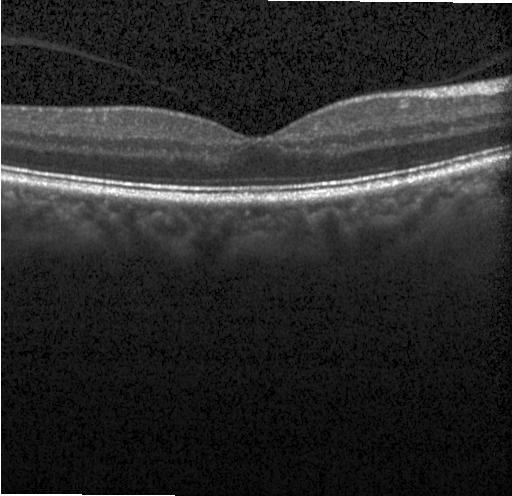 OCT line scan. Macular scan.
Diagnosis: neither choroidal neovascularization, diabetic macular edema, nor drusen.